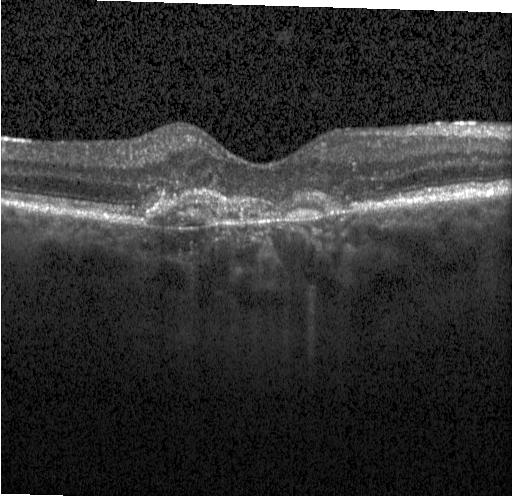
Diagnosis: choroidal neovascularization (CNV).